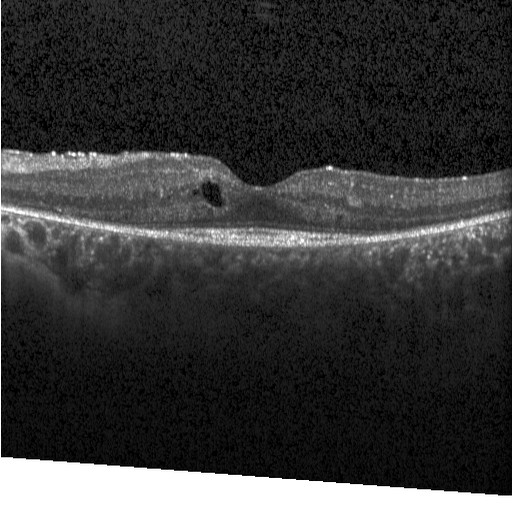
Impression: diabetic macular edema.